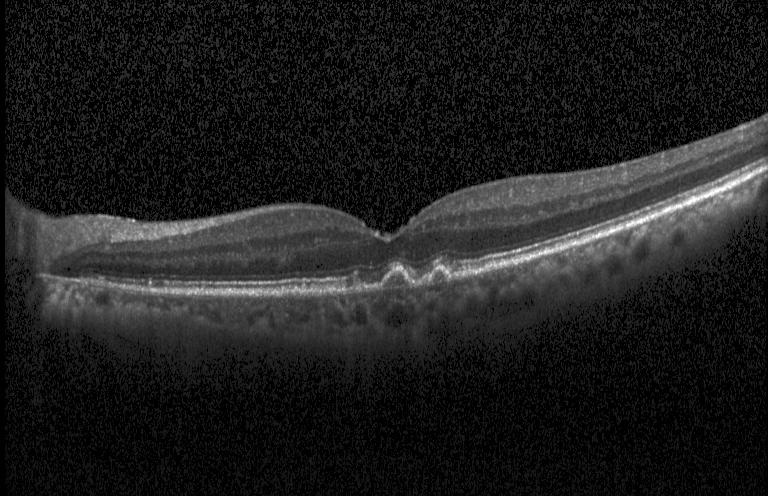
Optical coherence tomography B-scan.
OCT finding: drusen.